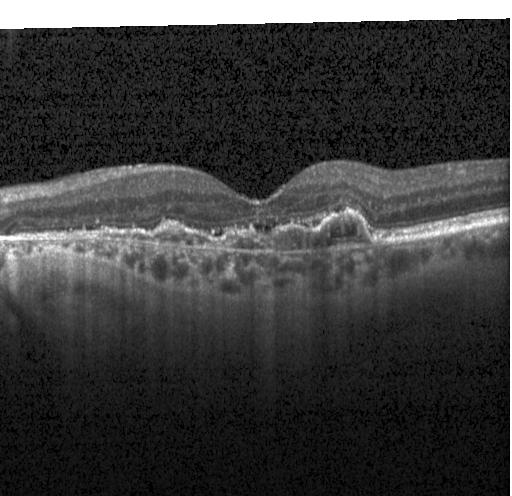
SD-OCT, retinal OCT cross-section, centered on the fovea, Heidelberg Spectralis OCT system
Impression: choroidal neovascularization (CNV).